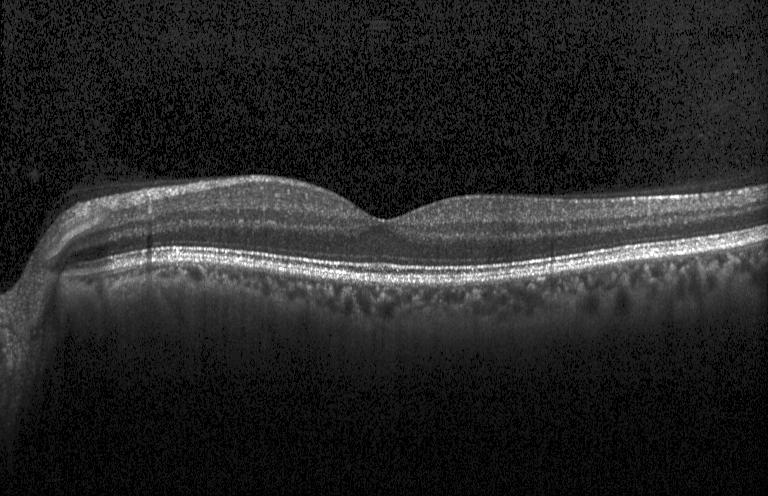
OCT line scan, horizontal scan through the fovea, Heidelberg Spectralis. Assessment: no choroidal neovascularization, diabetic macular edema, or drusen.